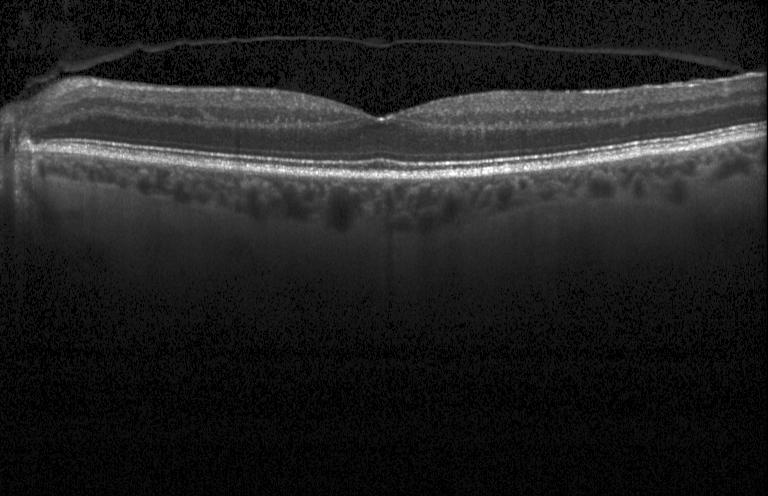 This B-scan demonstrates no CNV, no DME, and no drusen.